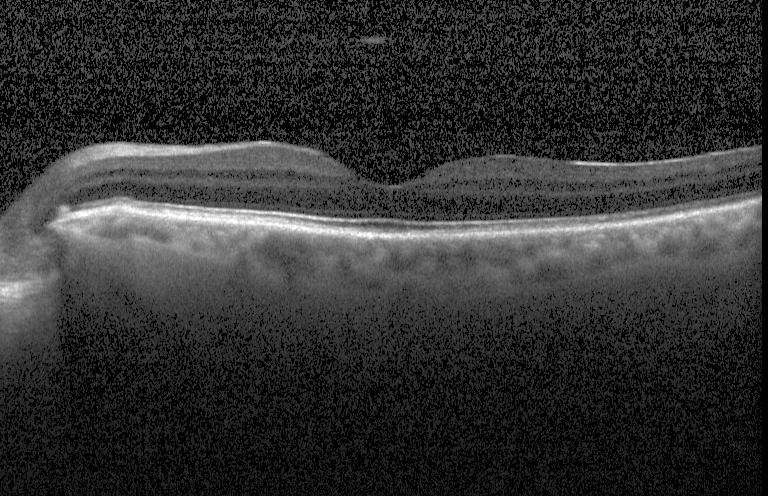
SD-OCT · optical coherence tomography B-scan — The scan shows neither CNV, DME, nor drusen.